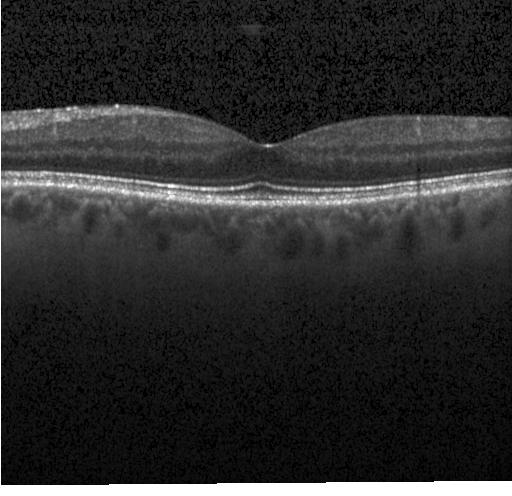
Macular OCT demonstrating no choroidal neovascularization, diabetic macular edema, or drusen.